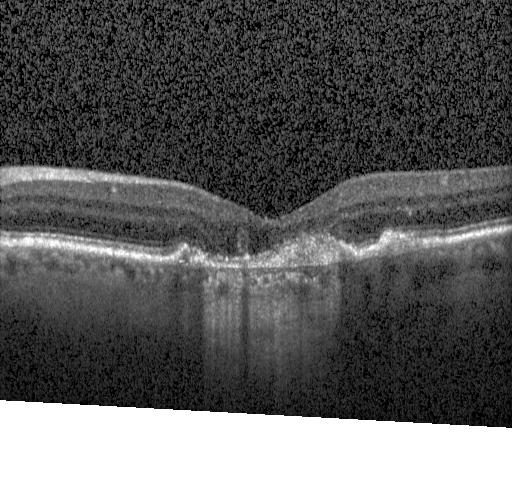 OCT line scan; instrument: Heidelberg Spectralis; centered on the fovea.
Assessment: choroidal neovascularization.